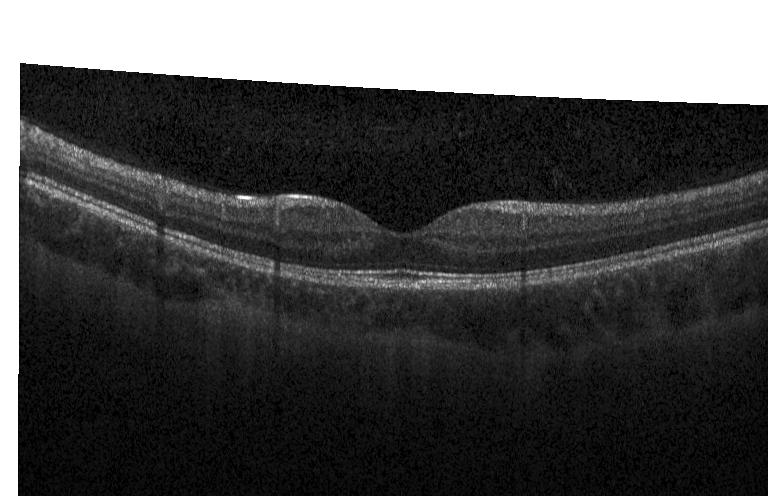
SD-OCT; OCT B-scan; Heidelberg Spectralis OCT system; through the macula.
This B-scan demonstrates neither choroidal neovascularization, diabetic macular edema, nor drusen.